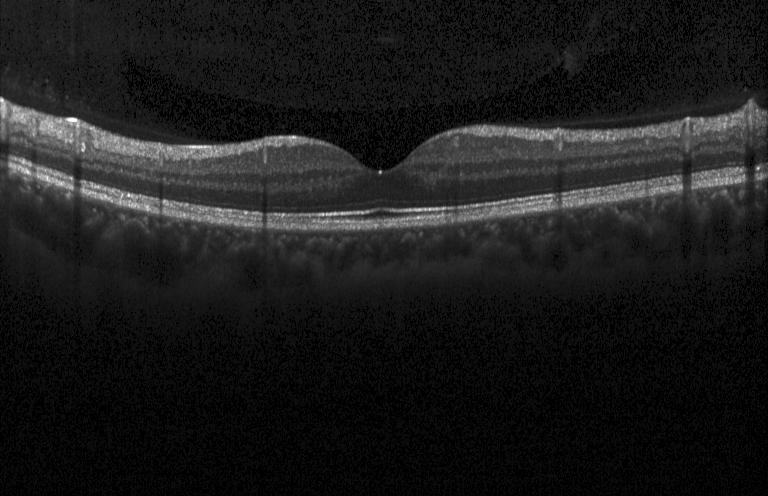 Macular scan · optical coherence tomography scan · instrument: Heidelberg Spectralis · SD-OCT — Dx: no choroidal neovascularization, diabetic macular edema, or drusen.